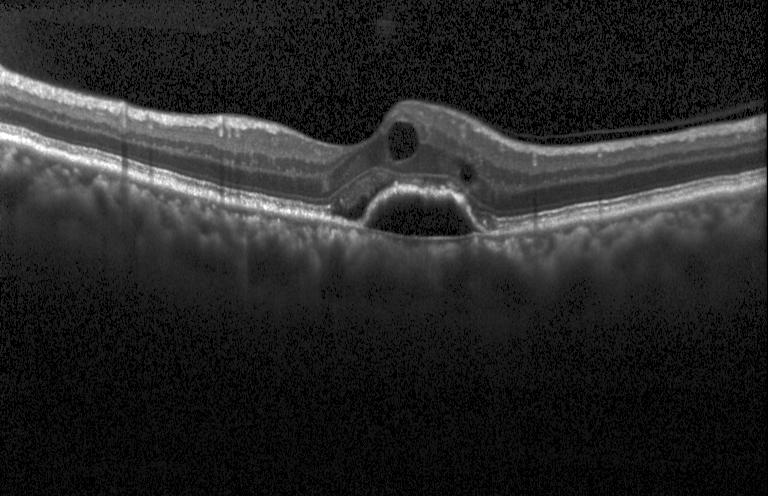 Acquired on a Heidelberg Spectralis; spectral-domain OCT; OCT B-scan; centered on the fovea. Choroidal neovascularization.